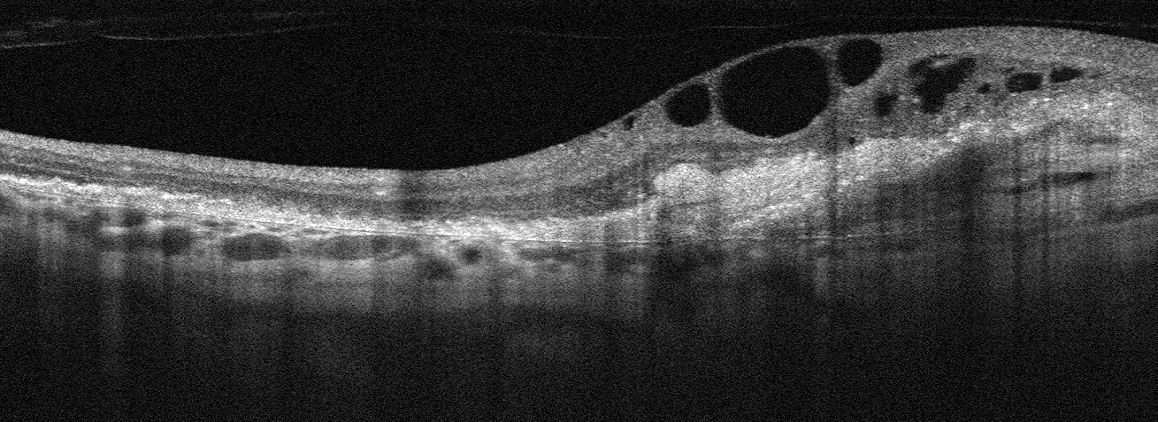
Right eye; optical coherence tomography scan.
Macular OCT: AMD.